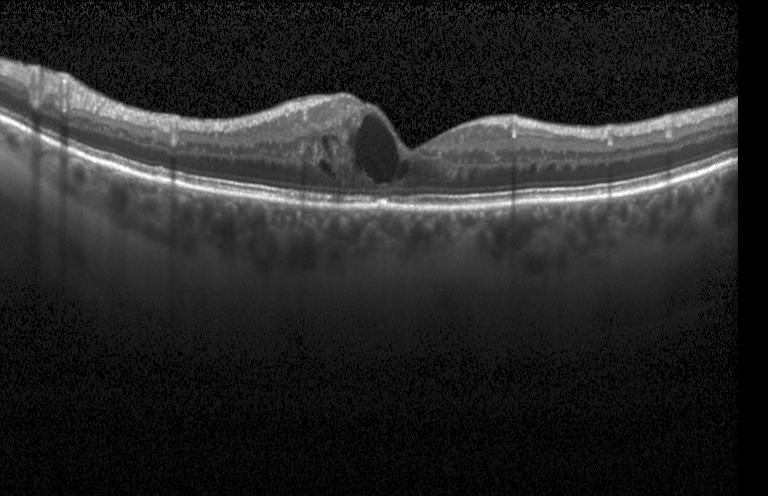

Spectral-domain OCT, optical coherence tomography scan.
The scan shows diabetic macular edema.